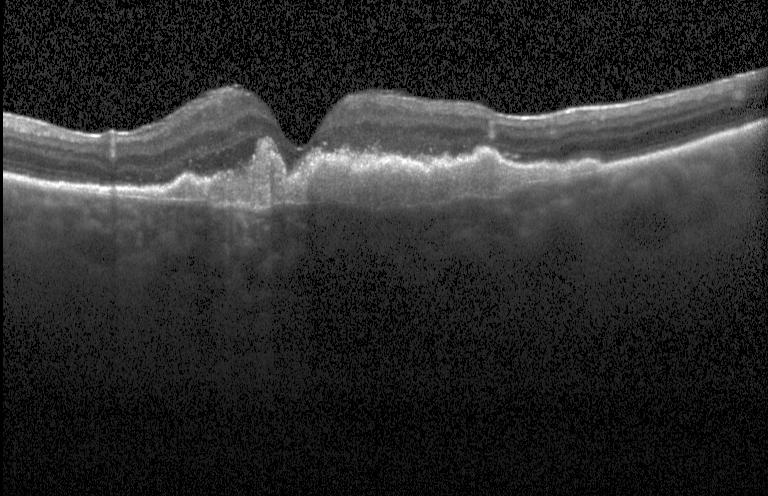
Retinal OCT B-scan, spectral-domain OCT.
Finding: choroidal neovascularization.